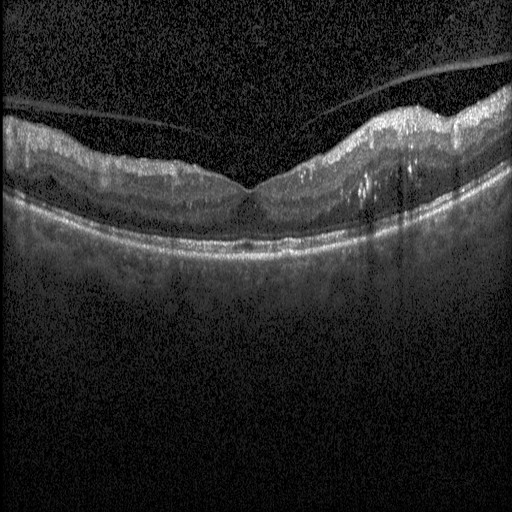

Macular OCT demonstrating diabetic macular edema.